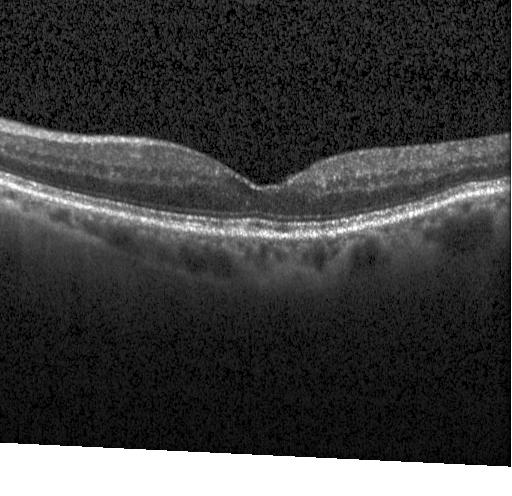
Retinal OCT B-scan · SD-OCT
Dx: no choroidal neovascularization, diabetic macular edema, or drusen.